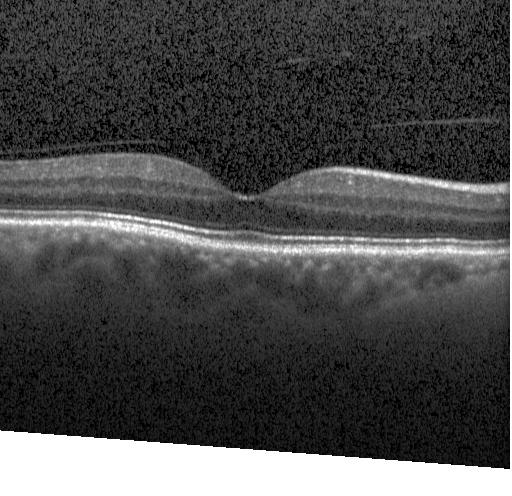
OCT B-scan; Heidelberg Spectralis — OCT finding: neither CNV, DME, nor drusen.